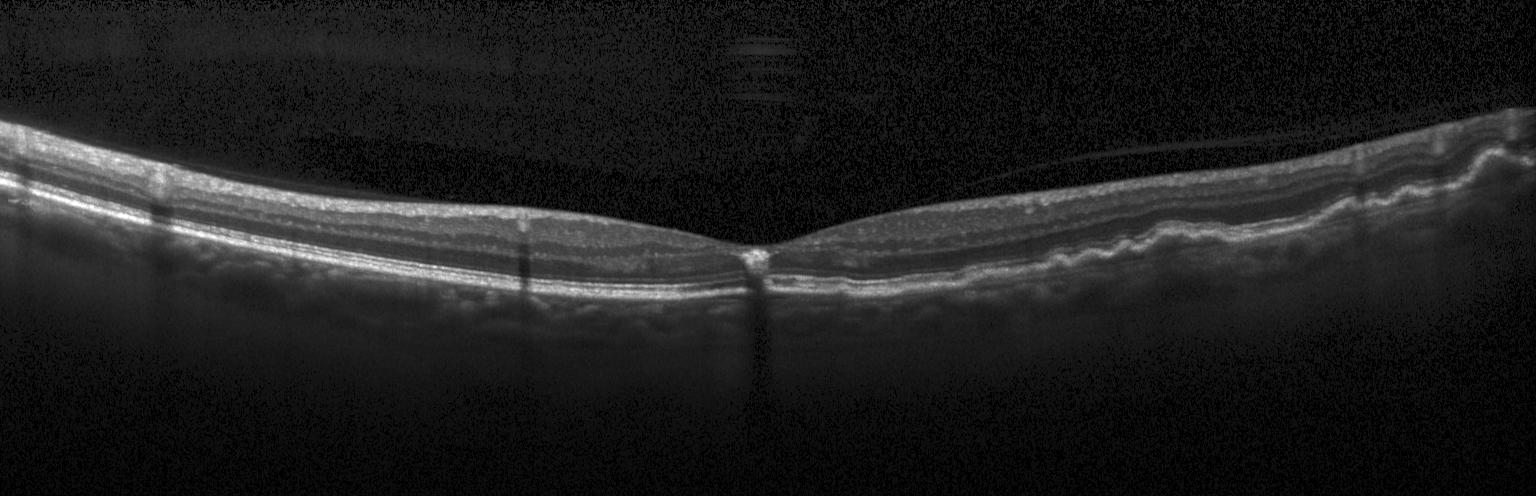

Acquired on a Heidelberg Spectralis. Spectral-domain optical coherence tomography. Retinal OCT B-scan. Fovea-centered. Diagnosis: a choroidal neovascular membrane.